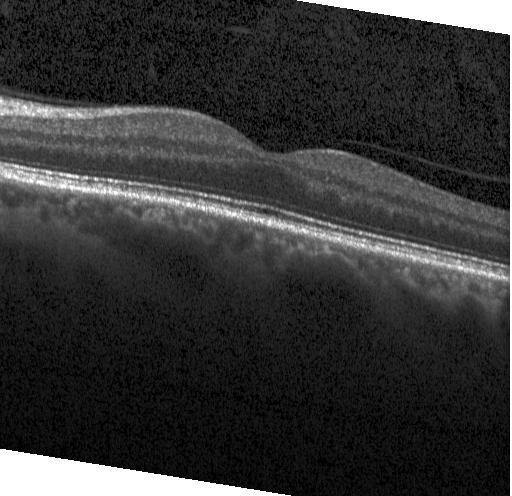
Dx: no evidence of choroidal neovascularization, diabetic macular edema, or drusen.